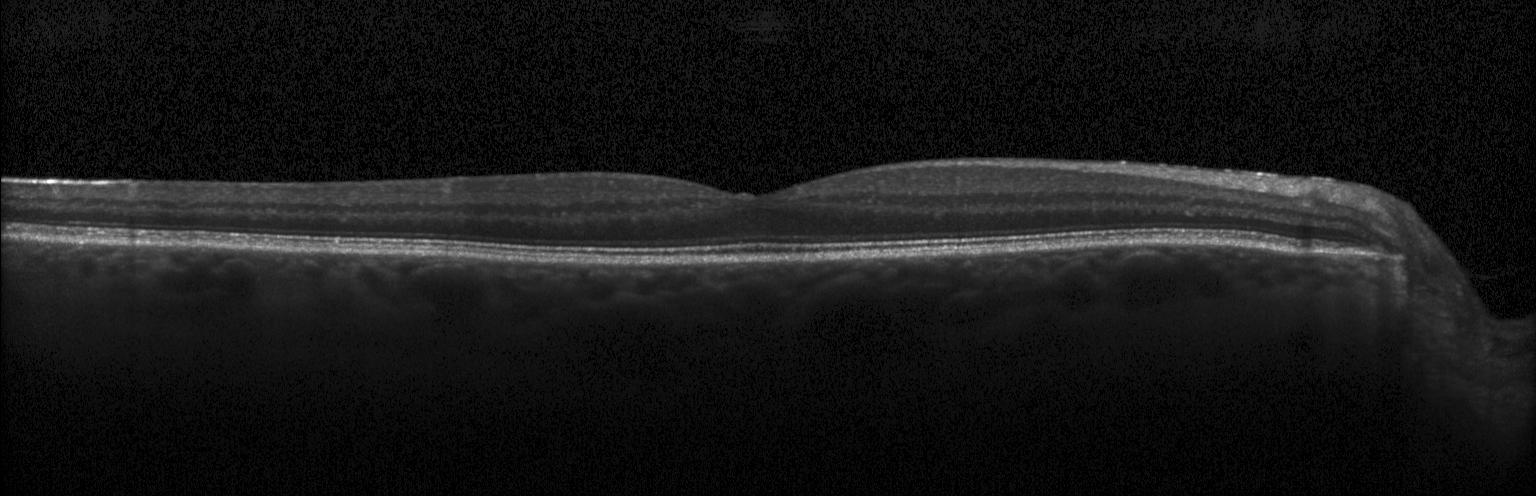
OCT B-scan. SD-OCT. Horizontal scan through the fovea. Heidelberg Spectralis OCT system. OCT finding: no CNV, no DME, and no drusen.